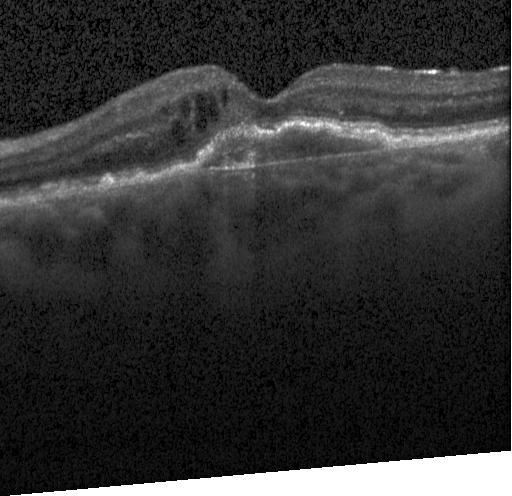 Optical coherence tomography scan; Heidelberg Spectralis
Impression: choroidal neovascularization (CNV).